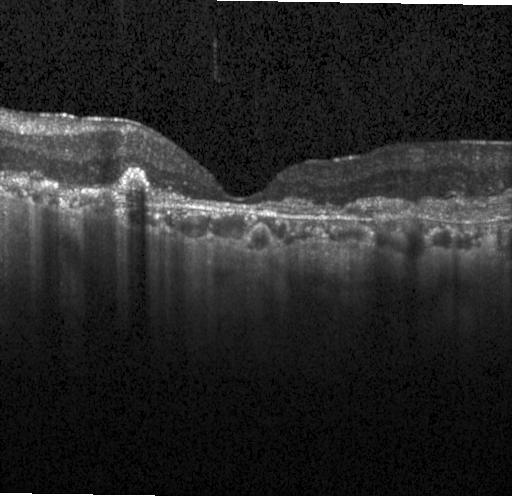 Macular OCT demonstrating a choroidal neovascular membrane.